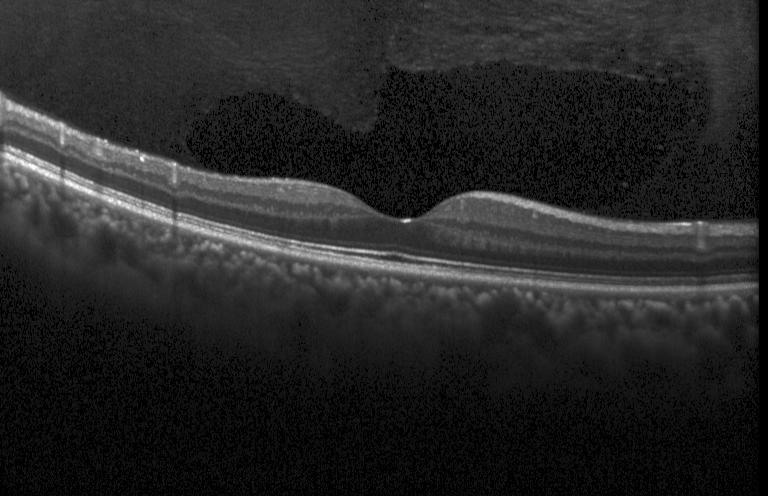 OCT scan showing no CNV, no DME, and no drusen.